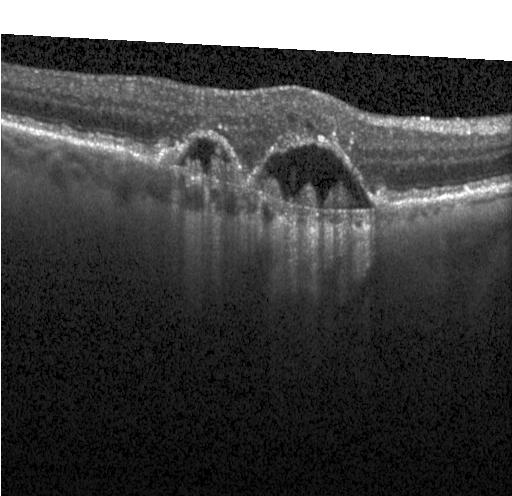 Assessment: choroidal neovascularization (CNV).